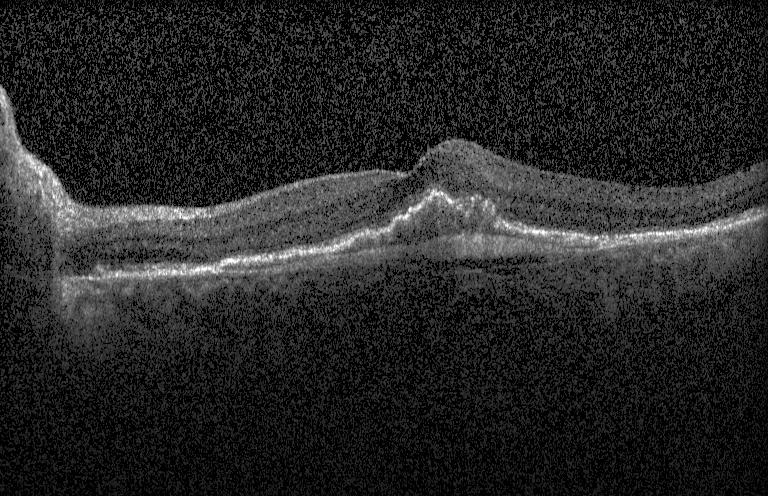
Optical coherence tomography B-scan — OCT finding: a choroidal neovascular membrane.